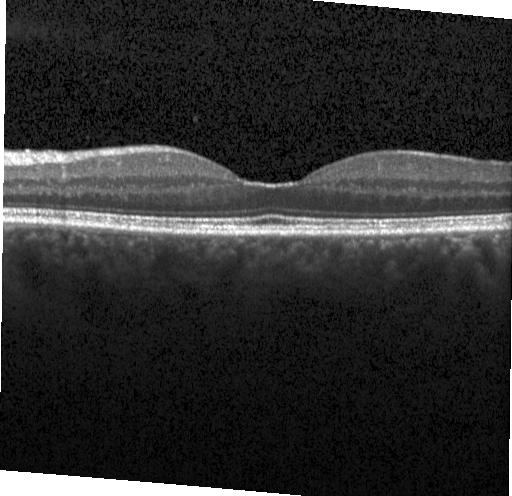 Macular OCT: no CNV, no DME, and no drusen.